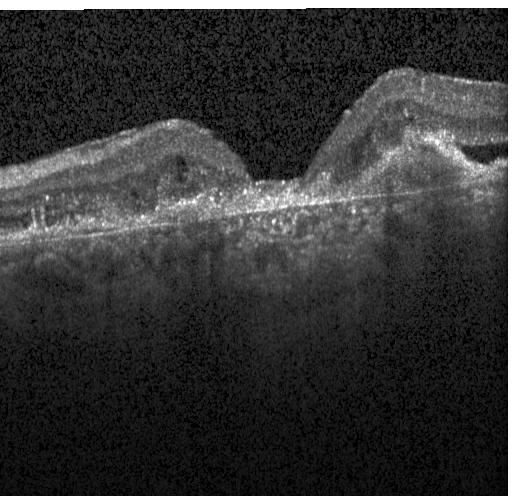 OCT B-scan. Acquired on a Heidelberg Spectralis. Spectral-domain OCT. This B-scan demonstrates a choroidal neovascular membrane.